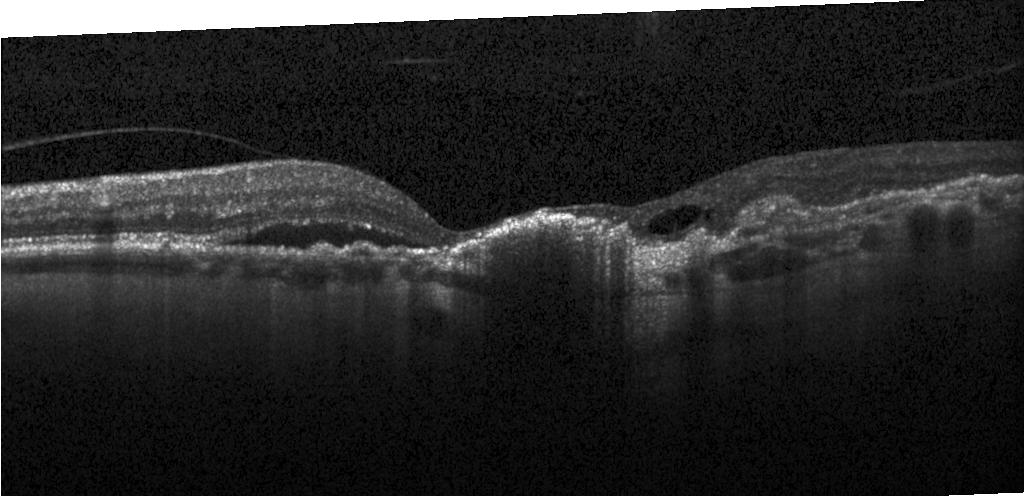

Retinal OCT cross-section showing a choroidal neovascular membrane.